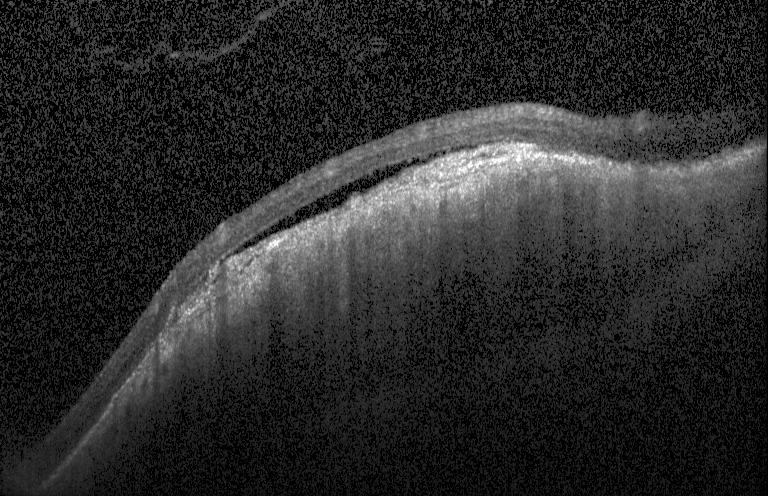
Optical coherence tomography scan. Impression: a choroidal neovascular membrane.